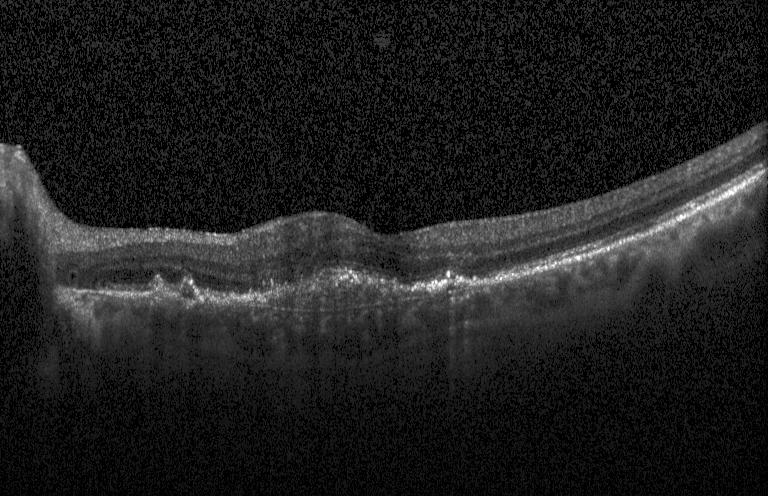
Optical coherence tomography B-scan — Impression: a choroidal neovascular membrane.